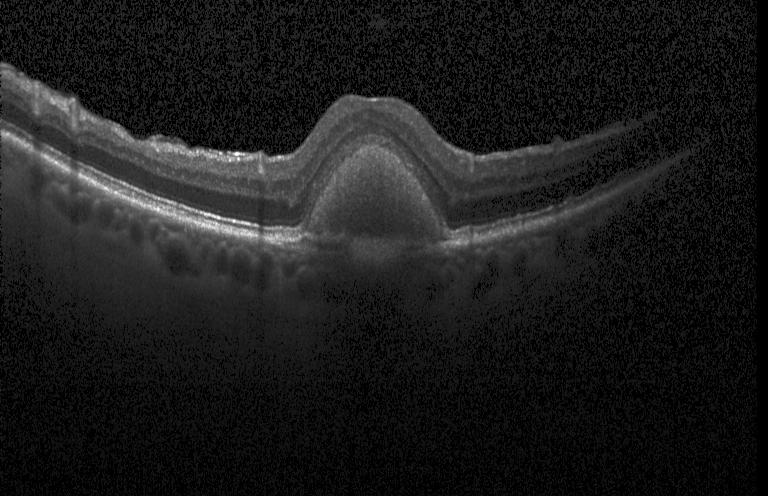 Horizontal scan through the fovea, retinal OCT cross-section, spectral-domain optical coherence tomography
The scan shows a choroidal neovascular membrane.